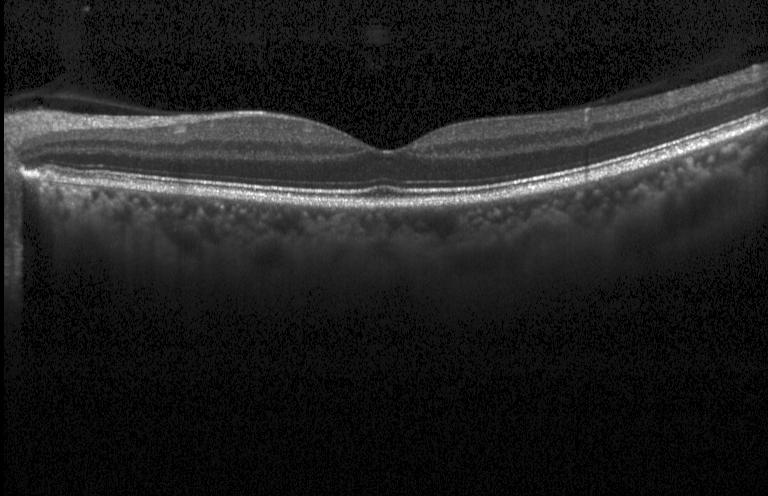 Centered on the fovea, optical coherence tomography B-scan — Assessment: neither CNV, DME, nor drusen.